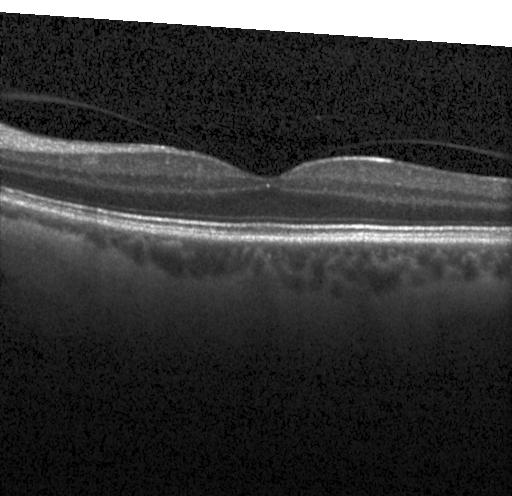 Heidelberg Spectralis; OCT B-scan.
Finding: no CNV, DME, or drusen.